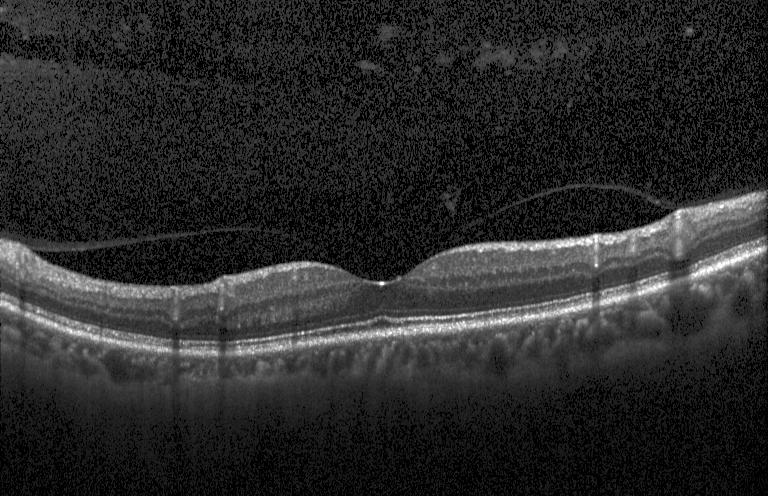
OCT finding: no choroidal neovascularization, diabetic macular edema, or drusen.